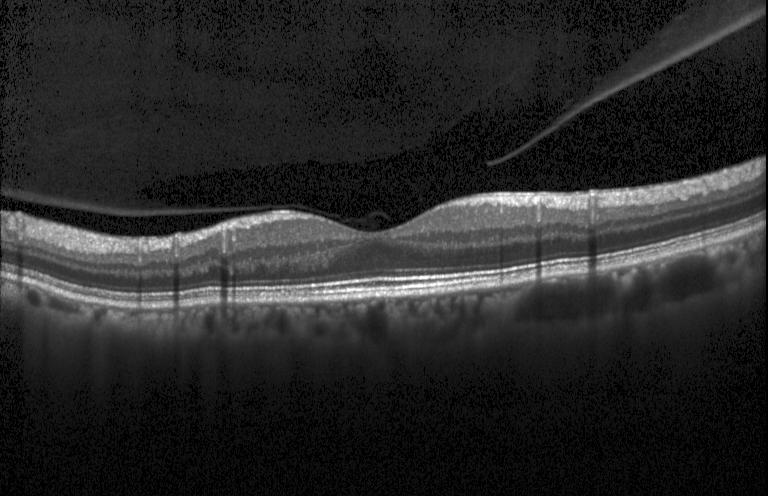

Macular scan; optical coherence tomography B-scan. Finding: no choroidal neovascularization, no diabetic macular edema, and no drusen.